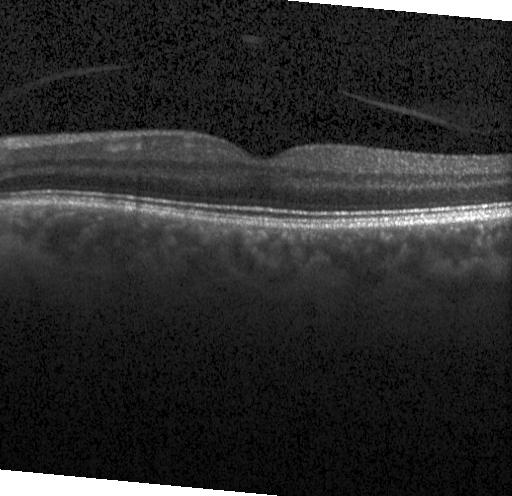

Retinal OCT cross-section.
Assessment: no choroidal neovascularization, diabetic macular edema, or drusen.